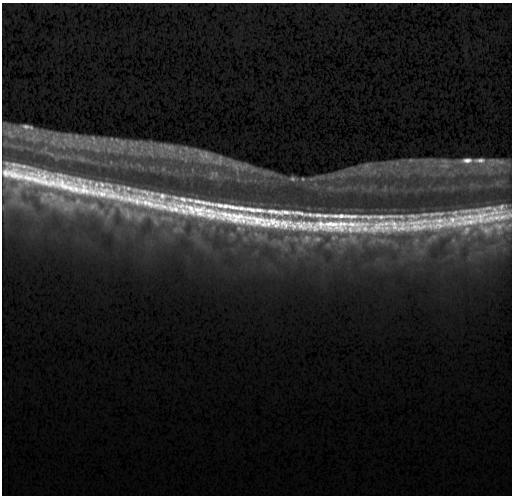

Spectral-domain OCT B-scan: no CNV, no DME, and no drusen.